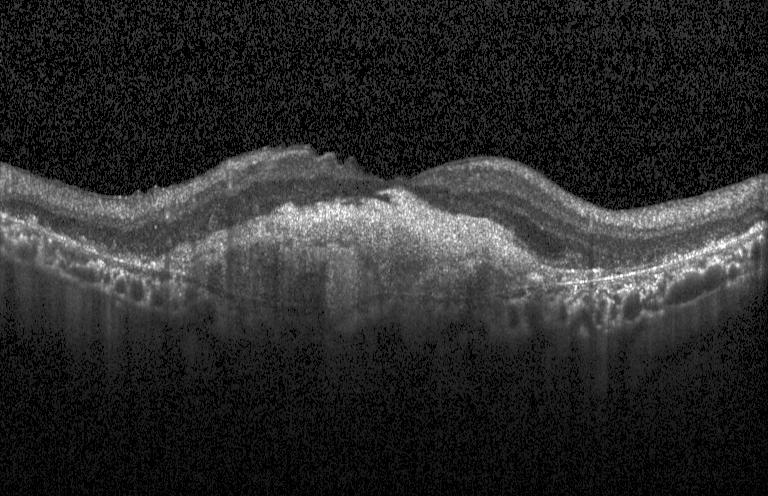

Instrument: Heidelberg Spectralis. Optical coherence tomography B-scan. Through the macula. Diagnosis: a choroidal neovascular membrane.